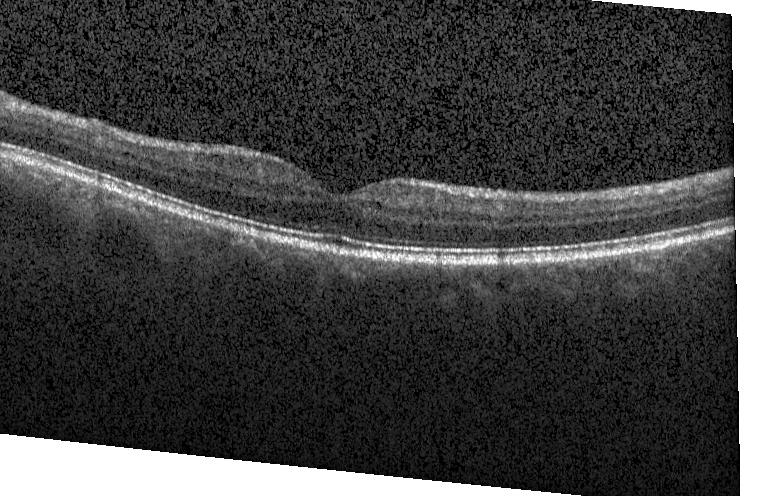
Retinal OCT cross-section showing no evidence of choroidal neovascularization, diabetic macular edema, or drusen.